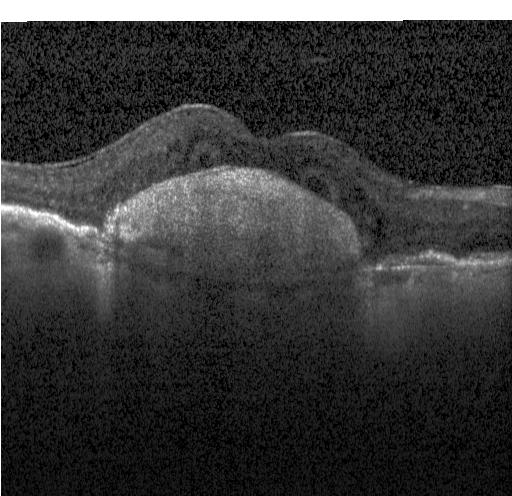
Macular scan · instrument: Heidelberg Spectralis · spectral-domain OCT · OCT line scan.
Choroidal neovascularization.